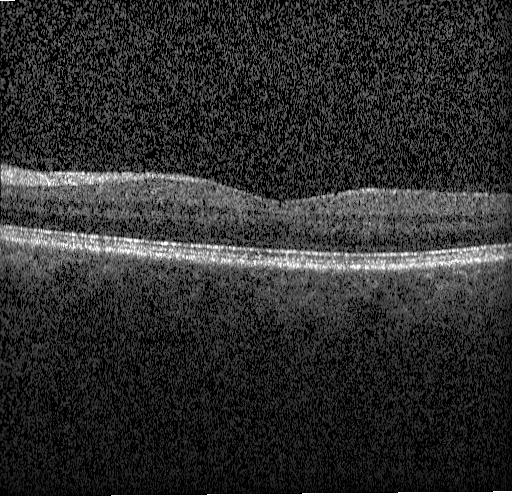

Optical coherence tomography scan, macular scan.
Dx: neither choroidal neovascularization, diabetic macular edema, nor drusen.